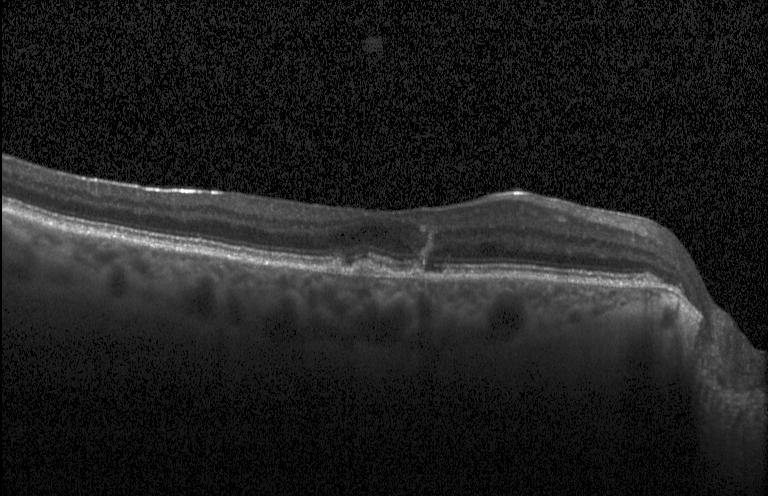
The scan shows drusen.